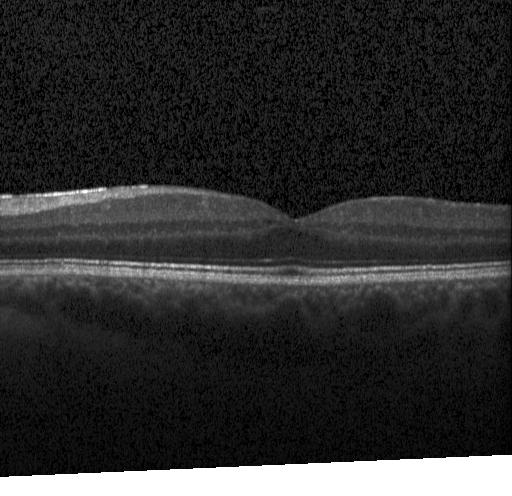
Centered on the fovea, instrument: Heidelberg Spectralis, spectral-domain optical coherence tomography, OCT line scan.
Dx: no choroidal neovascularization, no diabetic macular edema, and no drusen.